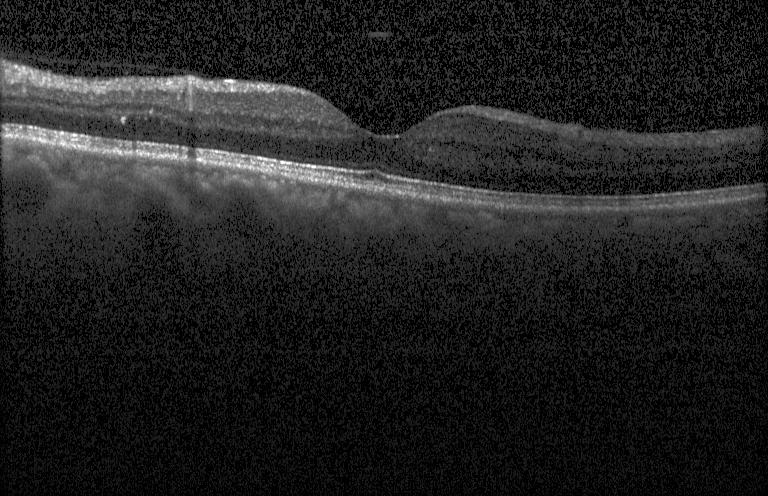
Finding: no CNV, DME, or drusen.